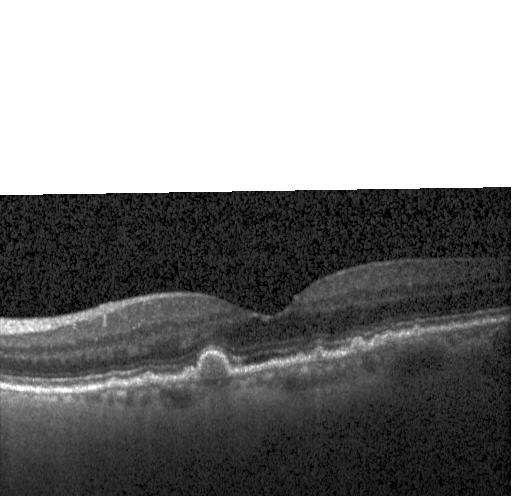 Fovea-centered · optical coherence tomography B-scan. Dx: drusen.